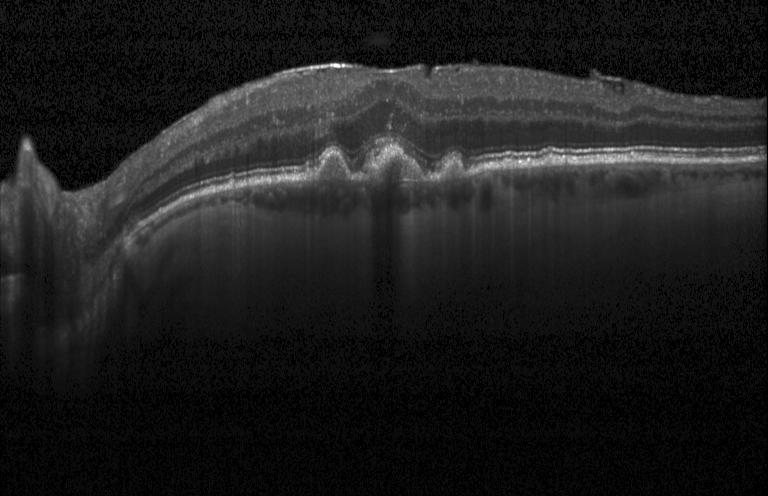
Horizontal scan through the fovea, OCT line scan
Finding: drusen.